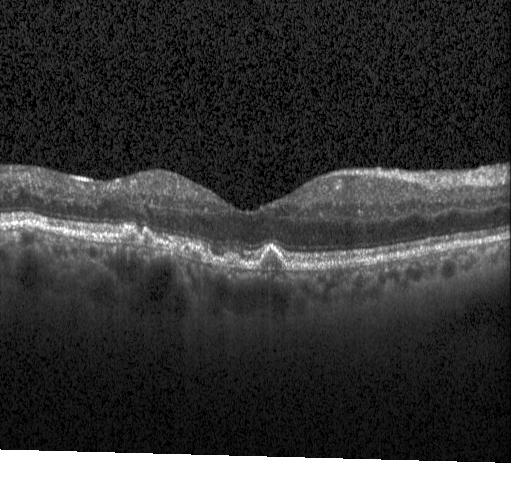 OCT line scan
Finding: drusen.